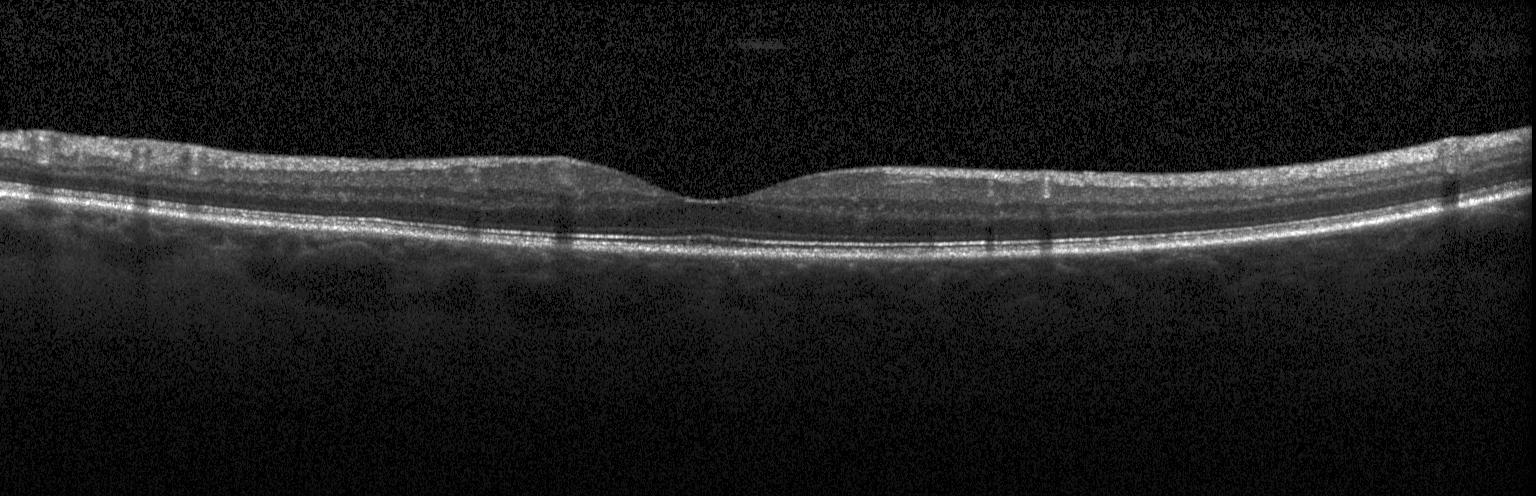 Retinal OCT cross-section. Acquired on a Heidelberg Spectralis — Neither choroidal neovascularization, diabetic macular edema, nor drusen.